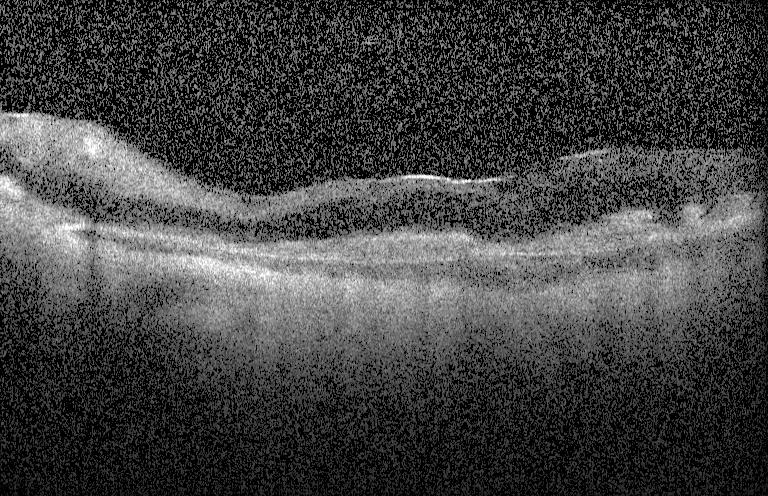
The scan shows choroidal neovascularization.